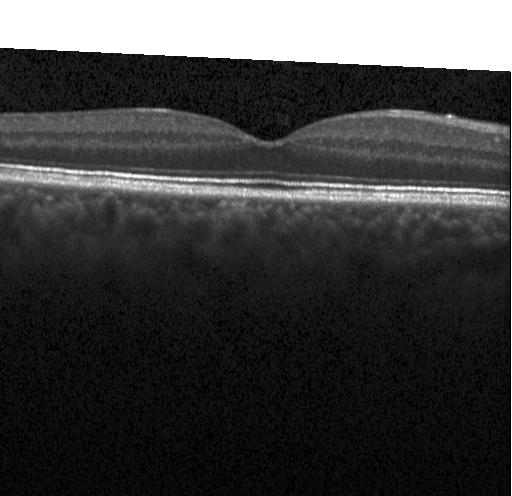
Heidelberg Spectralis OCT system. Optical coherence tomography scan — No evidence of choroidal neovascularization, diabetic macular edema, or drusen.